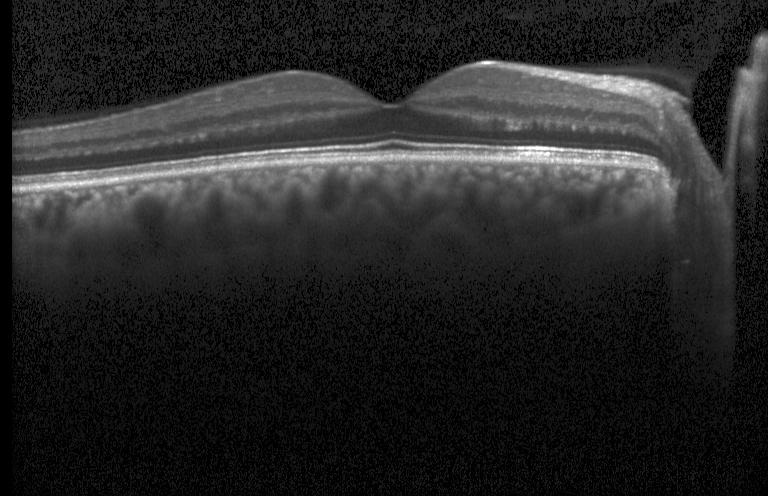

Spectral-domain OCT B-scan: no choroidal neovascularization, diabetic macular edema, or drusen.